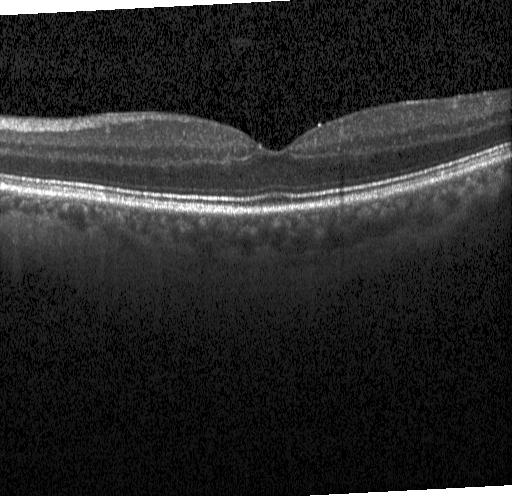 Heidelberg Spectralis, horizontal scan through the fovea, retinal OCT B-scan
This B-scan demonstrates no evidence of choroidal neovascularization, diabetic macular edema, or drusen.